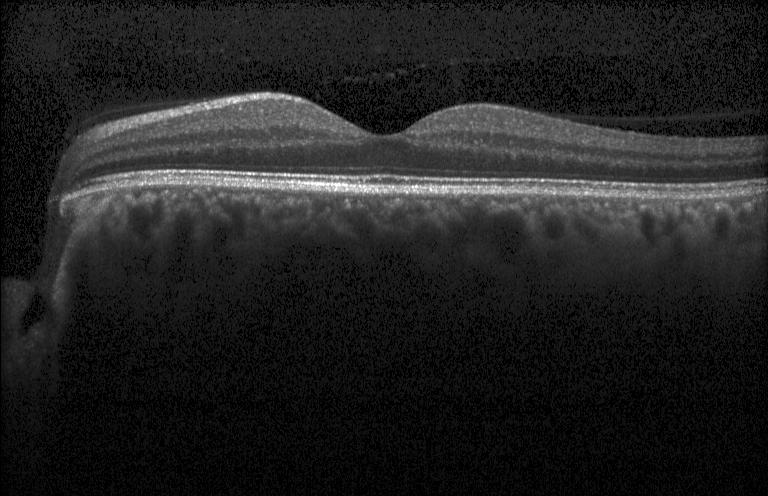
Spectral-domain optical coherence tomography. Macular scan. Optical coherence tomography scan. No evidence of choroidal neovascularization, diabetic macular edema, or drusen.